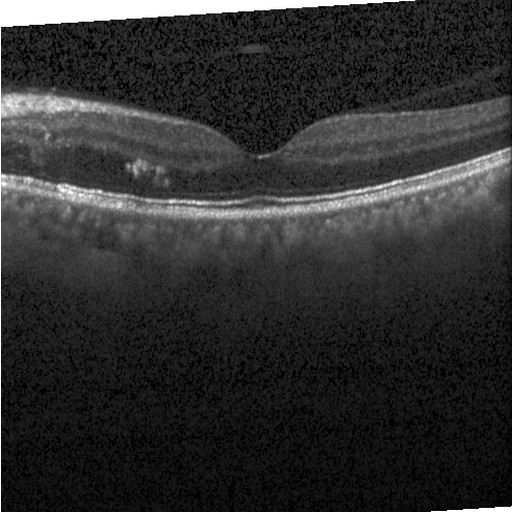
Spectral-domain optical coherence tomography · OCT line scan · Heidelberg Spectralis OCT system.
Diabetic macular edema.